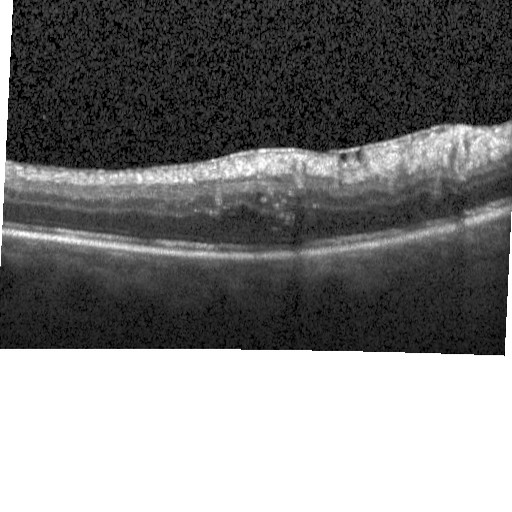 Macular OCT demonstrating diabetic macular edema (DME).